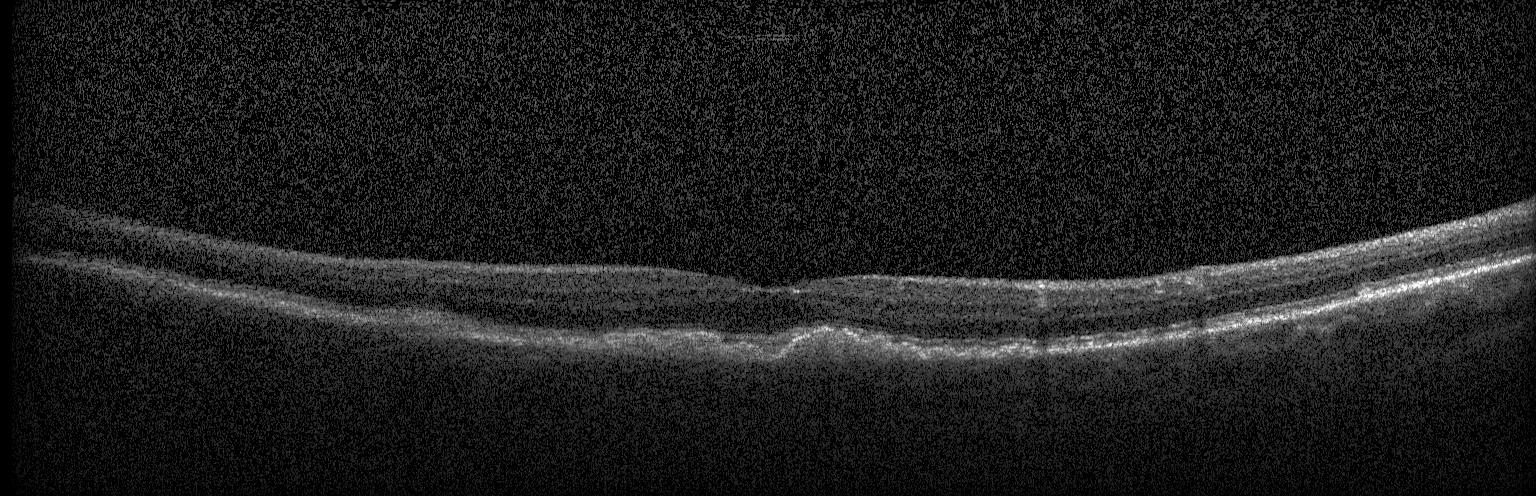

Optical coherence tomography B-scan; spectral-domain OCT.
Assessment: multiple drusen.